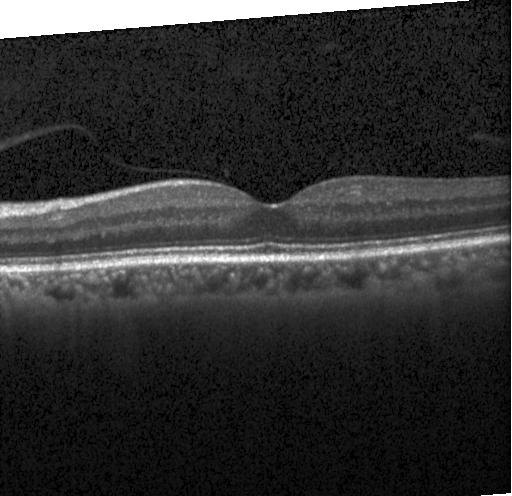
OCT B-scan. Diagnosis: no choroidal neovascularization, no diabetic macular edema, and no drusen.